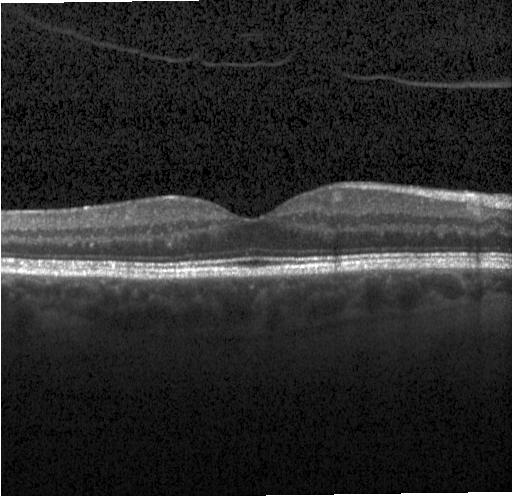

Centered on the fovea. Retinal OCT cross-section. Spectral-domain OCT
Finding: no choroidal neovascularization, no diabetic macular edema, and no drusen.